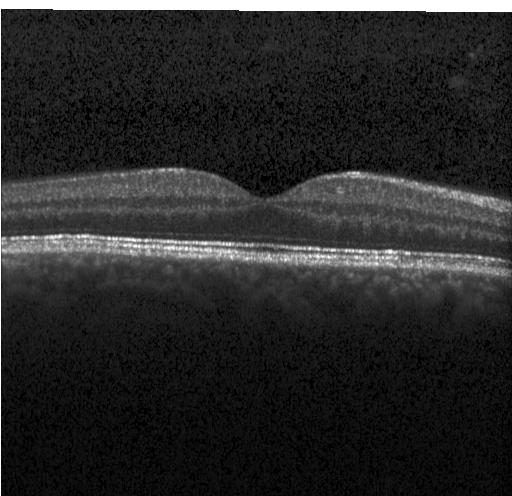 Assessment: neither CNV, DME, nor drusen.